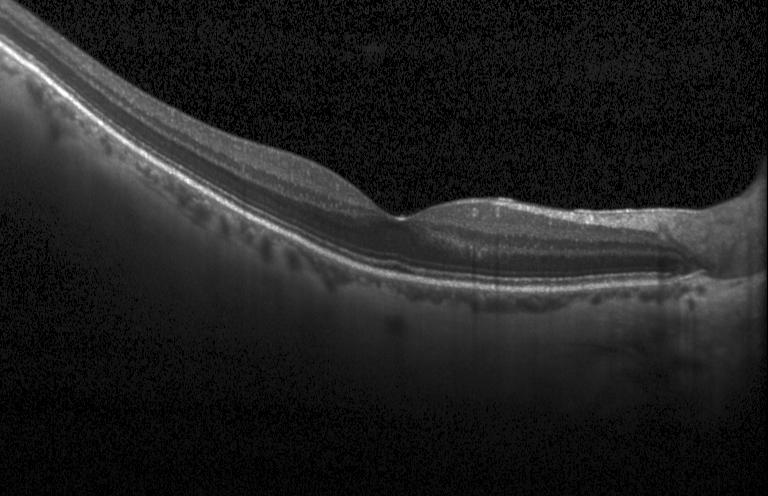
Assessment: no choroidal neovascularization, diabetic macular edema, or drusen.